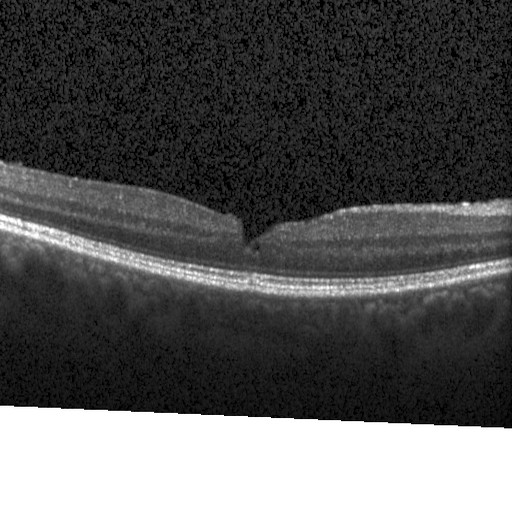
Impression: DME.